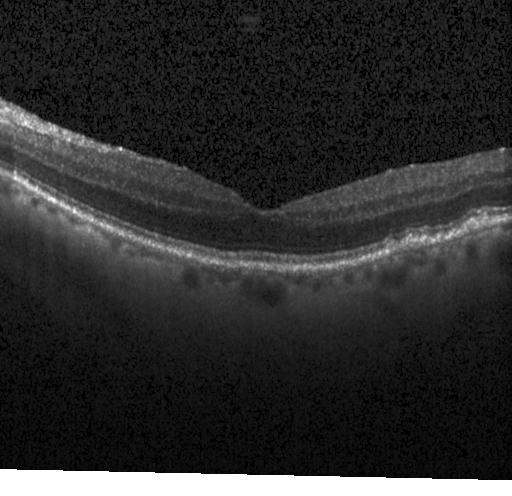
OCT line scan — Finding: sub-RPE drusenoid deposits.